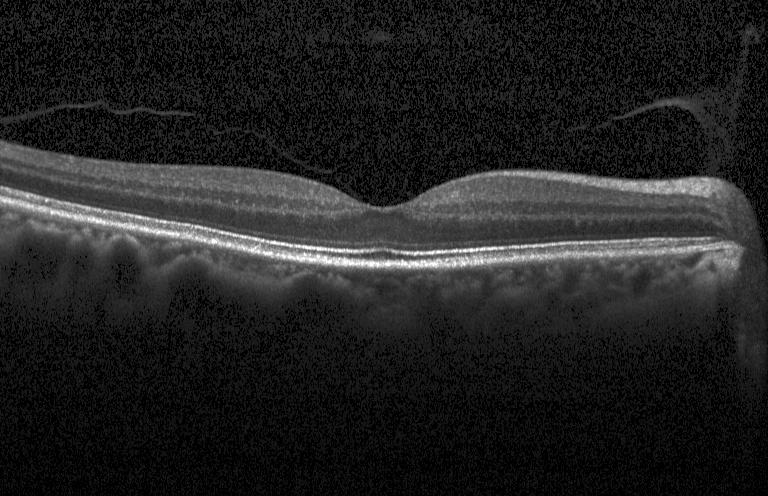 OCT finding: no choroidal neovascularization, no diabetic macular edema, and no drusen.